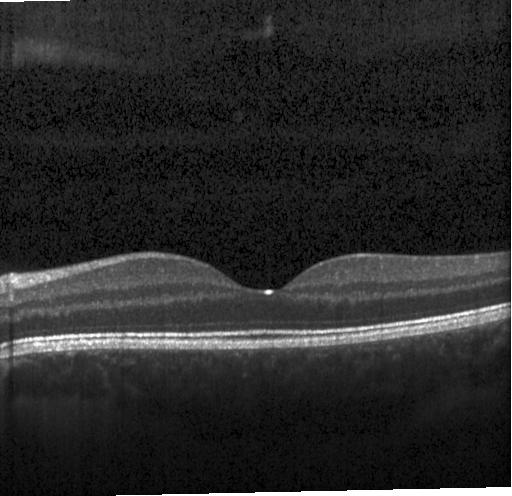

Macular OCT: no choroidal neovascularization, diabetic macular edema, or drusen.